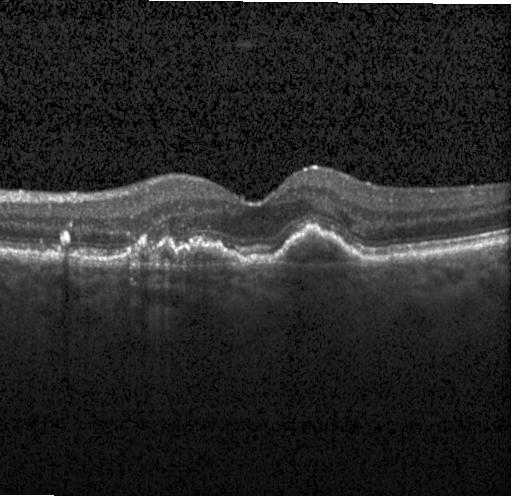
OCT finding: a choroidal neovascular membrane.